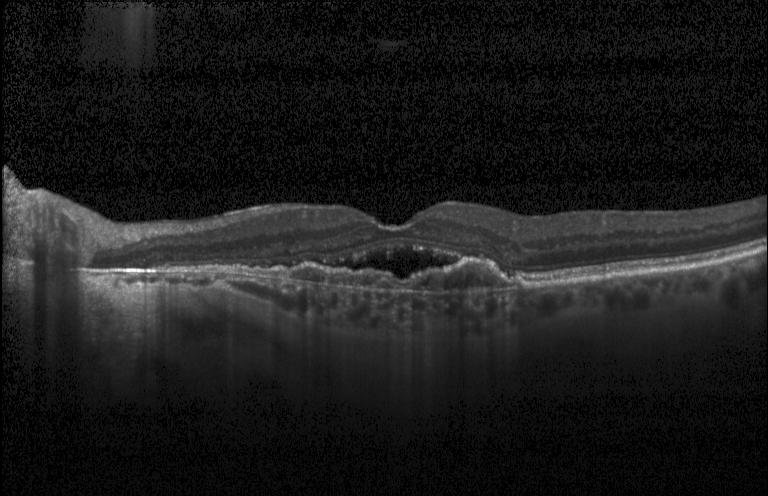 Macular OCT: a choroidal neovascular membrane.